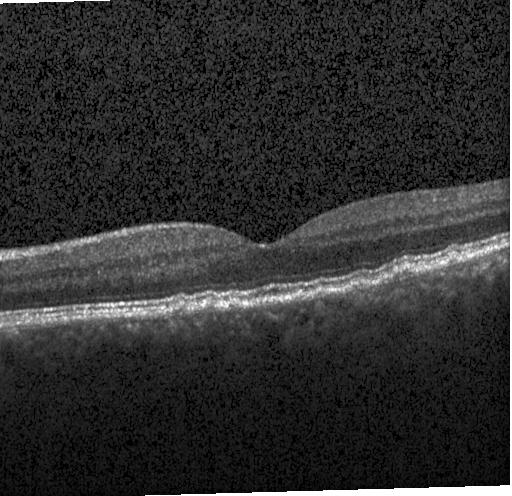 OCT line scan.
This B-scan demonstrates drusen.